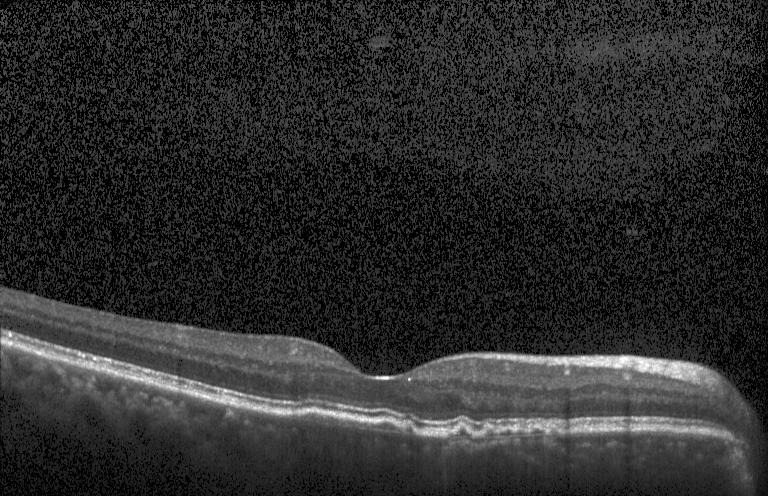

The scan shows drusen.